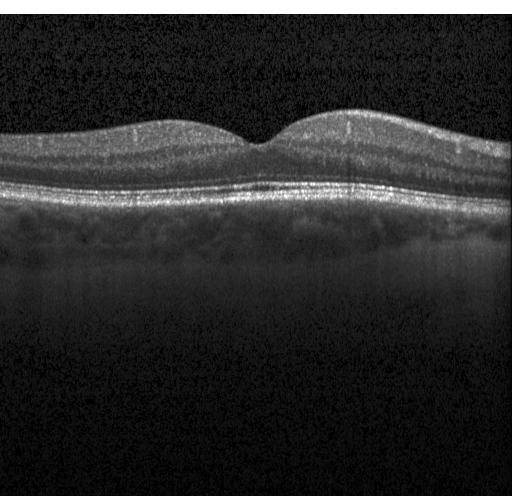 OCT line scan — Assessment: no choroidal neovascularization, diabetic macular edema, or drusen.